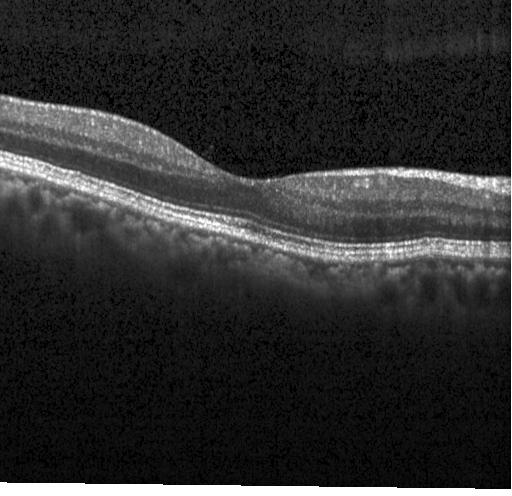

This B-scan demonstrates no choroidal neovascularization, no diabetic macular edema, and no drusen.